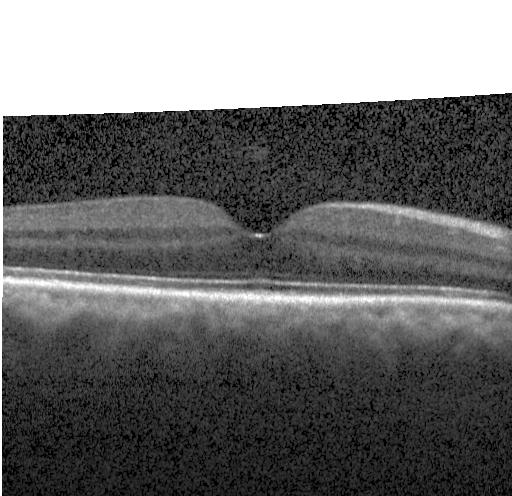 OCT finding: no evidence of choroidal neovascularization, diabetic macular edema, or drusen.